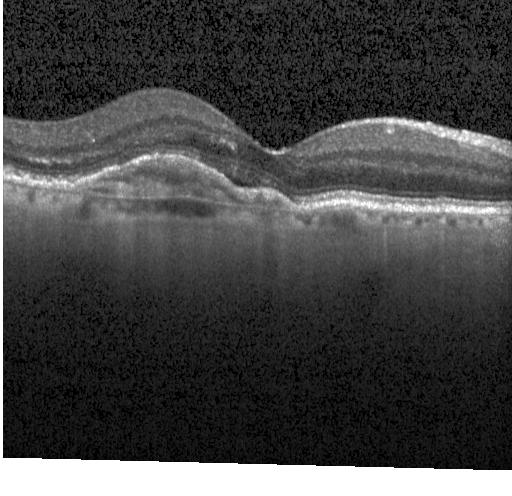 Macular scan · acquired on a Heidelberg Spectralis · OCT B-scan · spectral-domain optical coherence tomography — Impression: choroidal neovascularization.